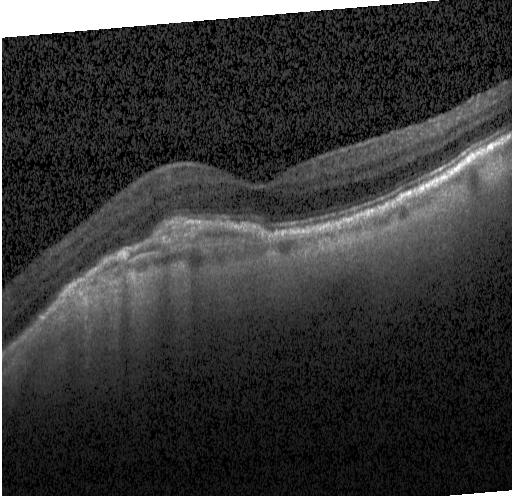

SD-OCT, Heidelberg Spectralis OCT system, optical coherence tomography B-scan.
The scan shows a choroidal neovascular membrane.